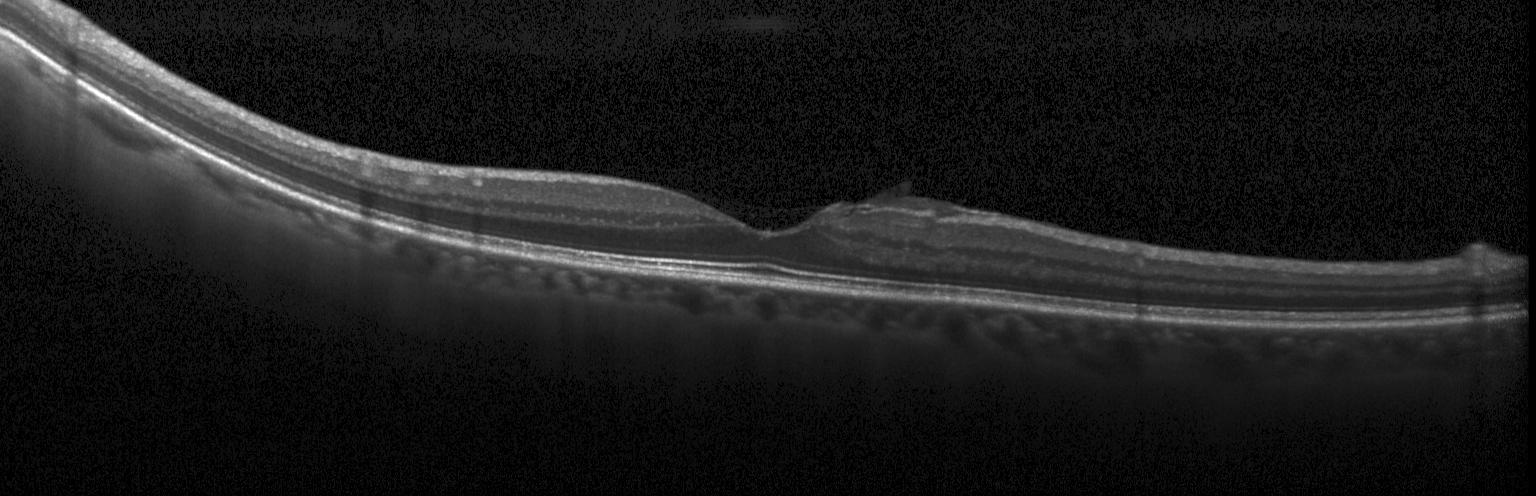
Spectral-domain OCT B-scan: neither choroidal neovascularization, diabetic macular edema, nor drusen.